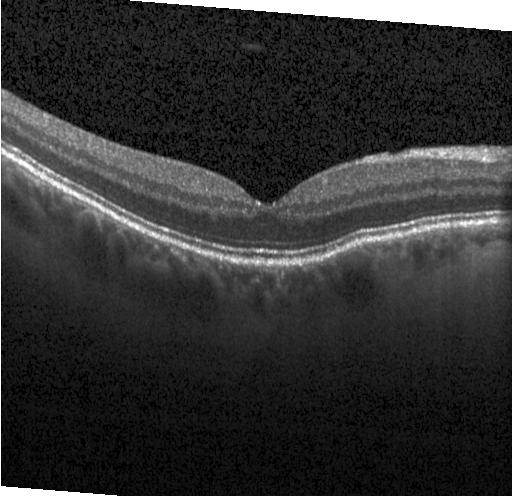 Dx: neither choroidal neovascularization, diabetic macular edema, nor drusen.